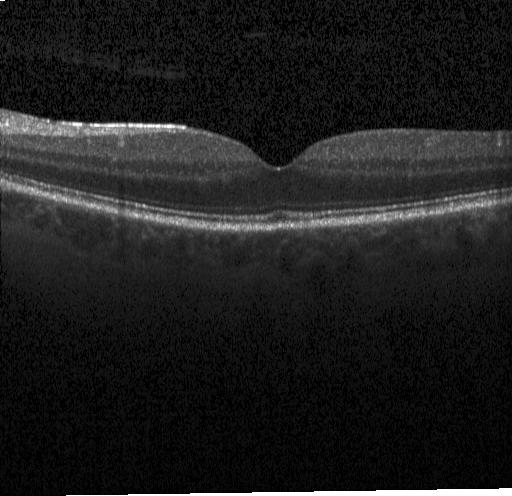

Centered on the fovea. Spectral-domain optical coherence tomography. Optical coherence tomography B-scan
Diagnosis: no evidence of choroidal neovascularization, diabetic macular edema, or drusen.